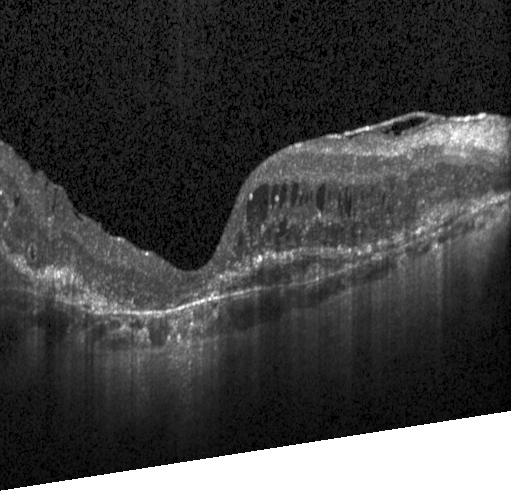
OCT line scan. Fovea-centered.
The scan shows a choroidal neovascular membrane.